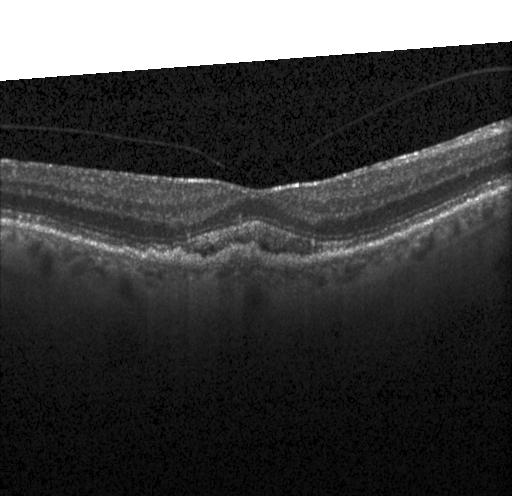

Optical coherence tomography B-scan; spectral-domain optical coherence tomography; fovea-centered; acquired on a Heidelberg Spectralis — Diagnosis: a choroidal neovascular membrane.